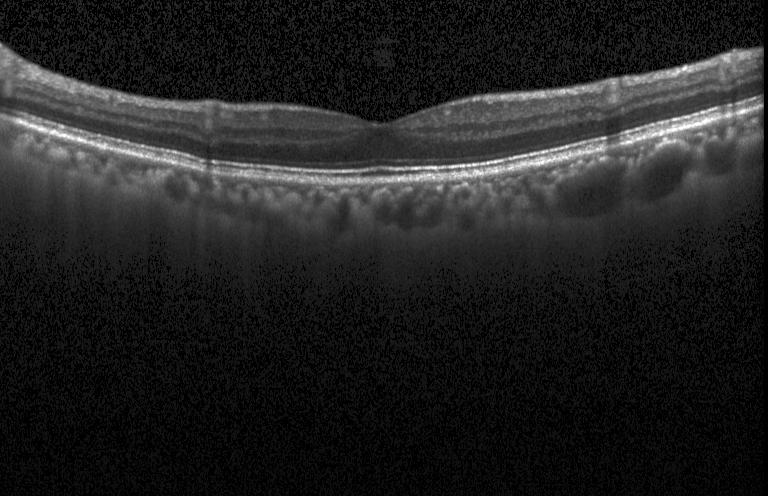 Centered on the fovea · instrument: Heidelberg Spectralis · spectral-domain OCT · retinal OCT cross-section
This B-scan demonstrates no evidence of choroidal neovascularization, diabetic macular edema, or drusen.